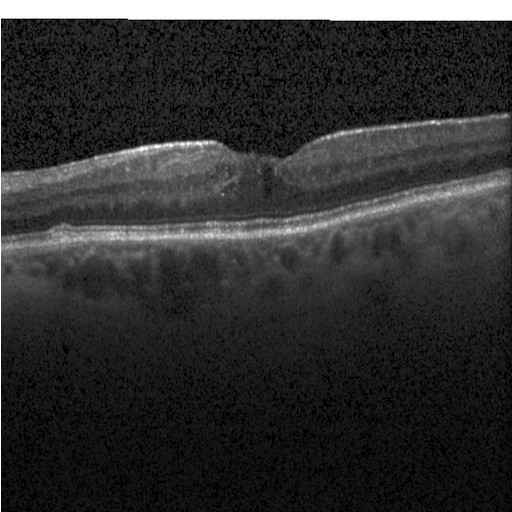
Optical coherence tomography B-scan, SD-OCT
Diabetic macular edema.